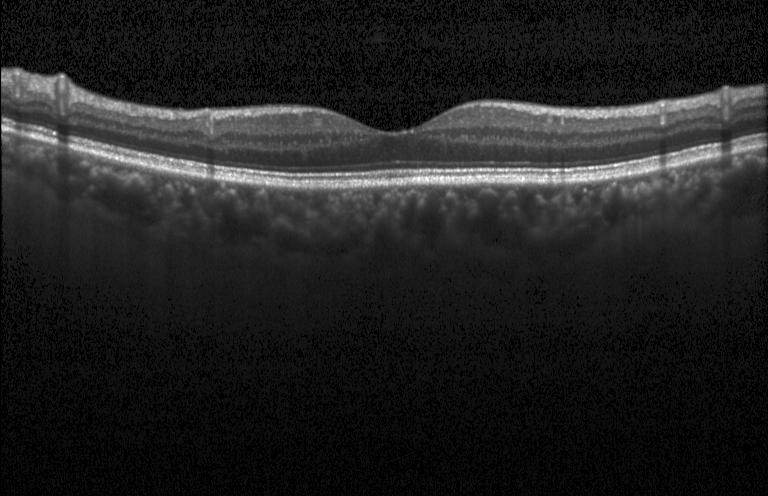 Spectral-domain optical coherence tomography · OCT line scan.
Dx: no evidence of choroidal neovascularization, diabetic macular edema, or drusen.